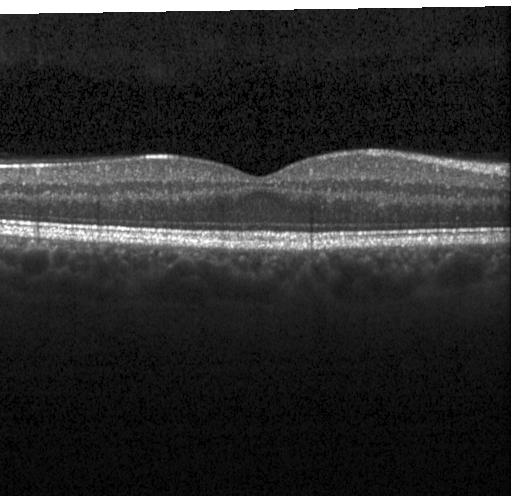
Instrument: Heidelberg Spectralis · spectral-domain OCT · optical coherence tomography B-scan. Diagnosis: no evidence of CNV, DME, or drusen.